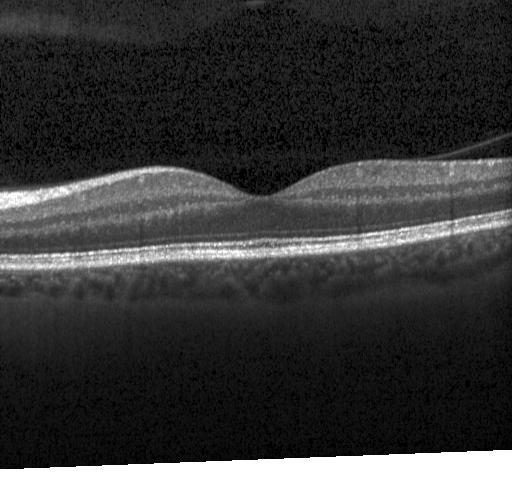

The scan shows no evidence of choroidal neovascularization, diabetic macular edema, or drusen.